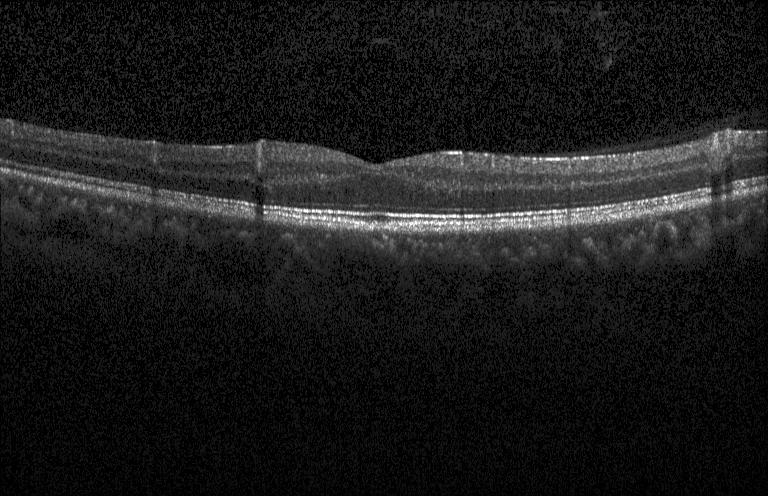
Acquired on a Heidelberg Spectralis, spectral-domain optical coherence tomography, OCT line scan, through the macula
Diagnosis: no CNV, DME, or drusen.